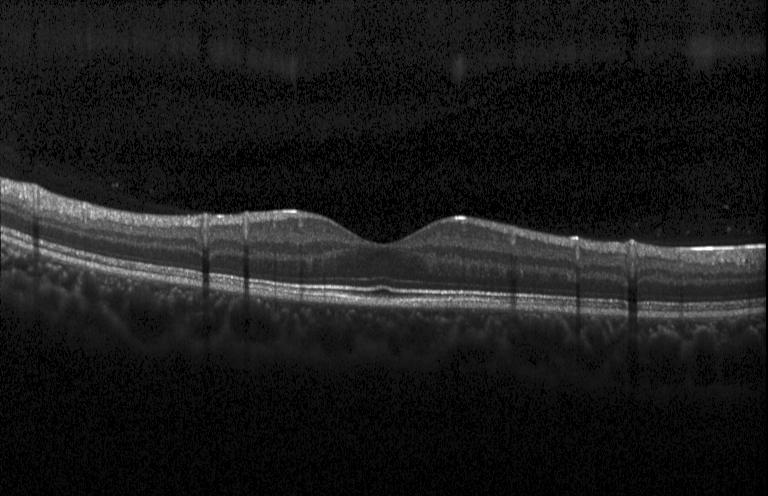
SD-OCT; optical coherence tomography scan. This B-scan demonstrates no CNV, no DME, and no drusen.